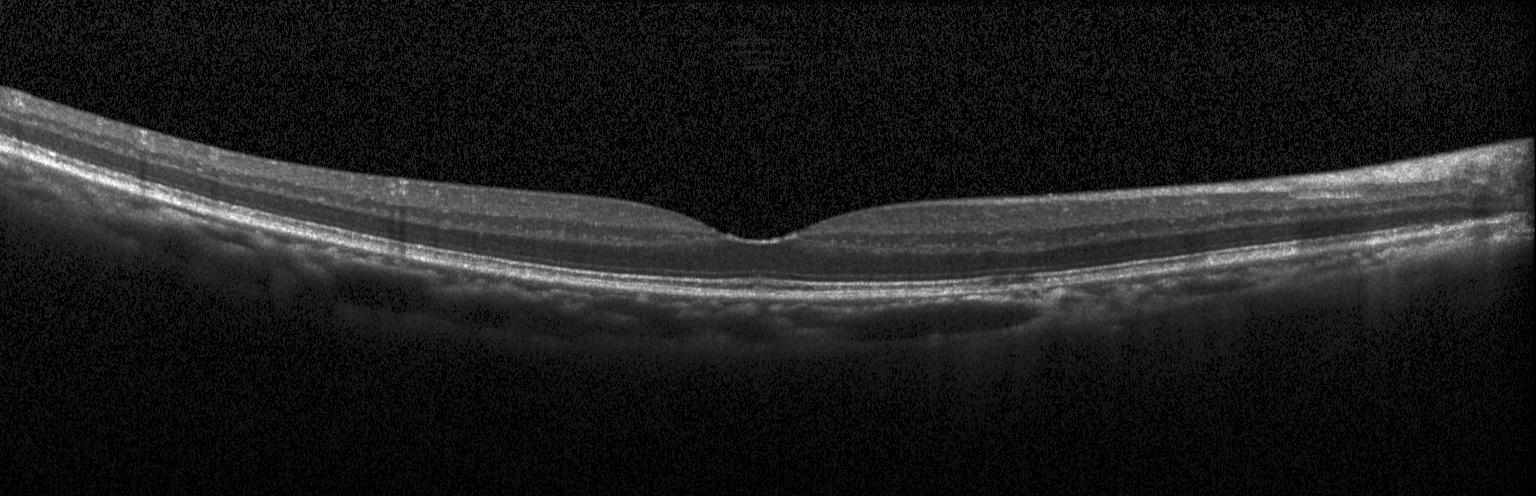 SD-OCT · retinal OCT B-scan
Dx: no choroidal neovascularization, no diabetic macular edema, and no drusen.